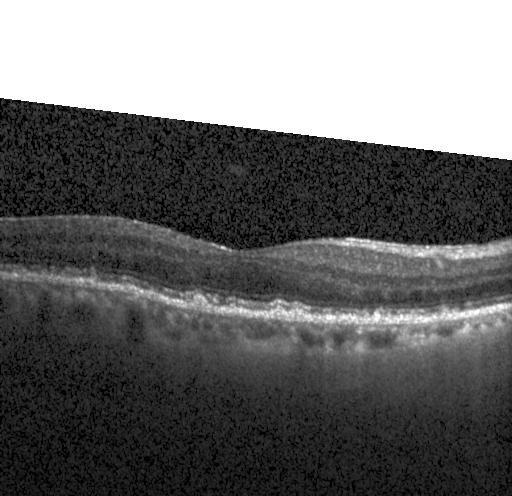 Retinal OCT cross-section.
Dx: drusen.